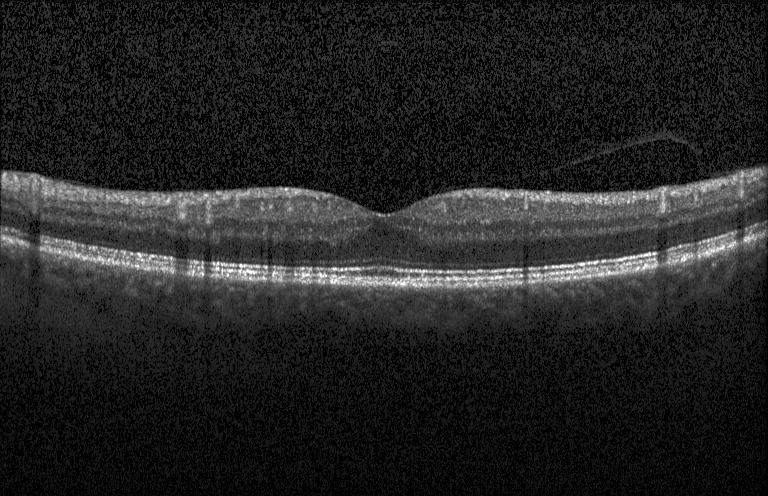 OCT B-scan. Spectral-domain OCT. Horizontal scan through the fovea. Heidelberg Spectralis — Diagnosis: no choroidal neovascularization, diabetic macular edema, or drusen.